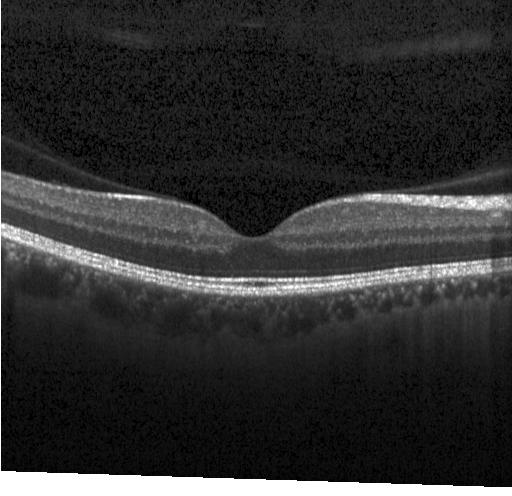

Spectral-domain OCT B-scan: neither CNV, DME, nor drusen.